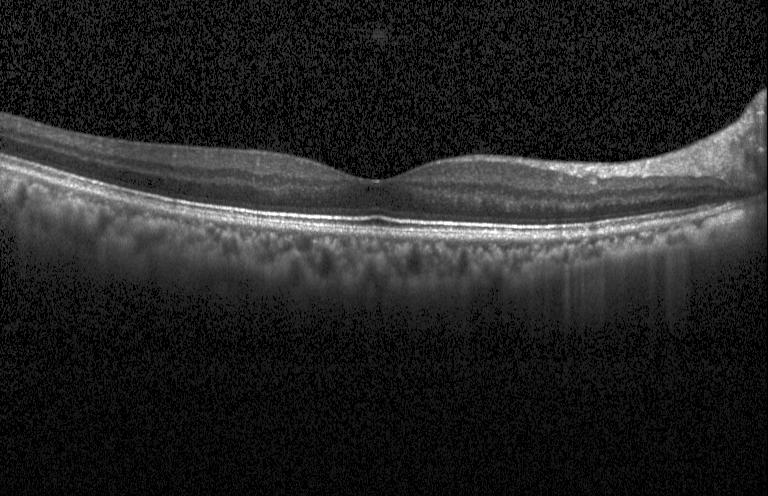 Finding: no choroidal neovascularization, no diabetic macular edema, and no drusen.